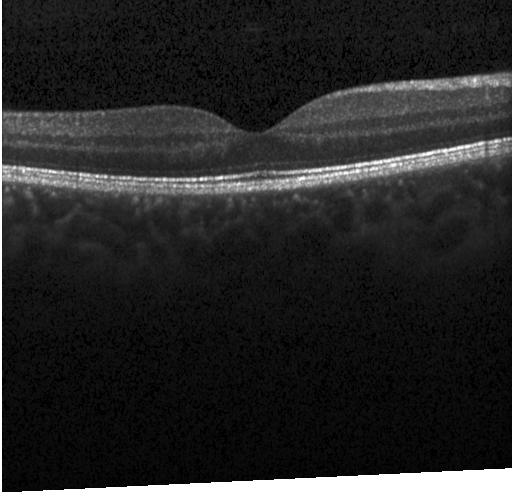

Optical coherence tomography B-scan; Heidelberg Spectralis OCT system.
Assessment: no choroidal neovascularization, no diabetic macular edema, and no drusen.